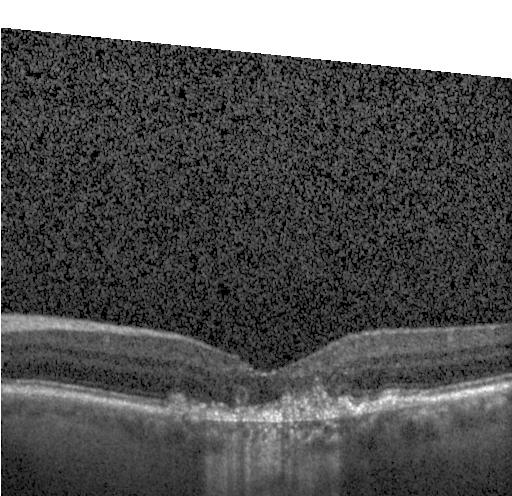

Instrument: Heidelberg Spectralis; OCT line scan; through the macula; SD-OCT. This B-scan demonstrates a choroidal neovascular membrane.